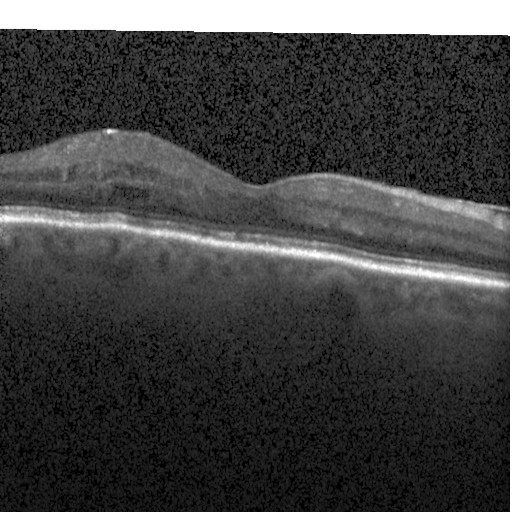 The scan shows DME.